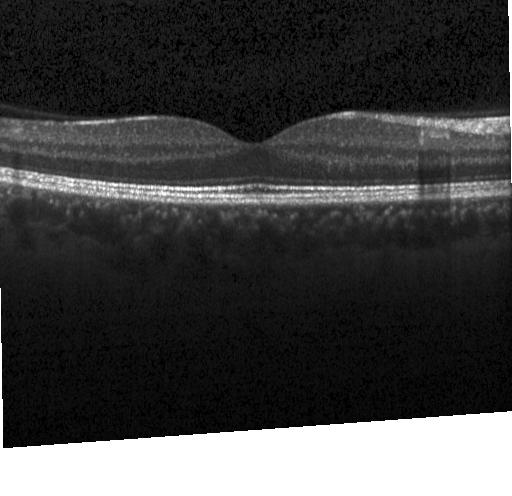

Macular OCT: no choroidal neovascularization, no diabetic macular edema, and no drusen.